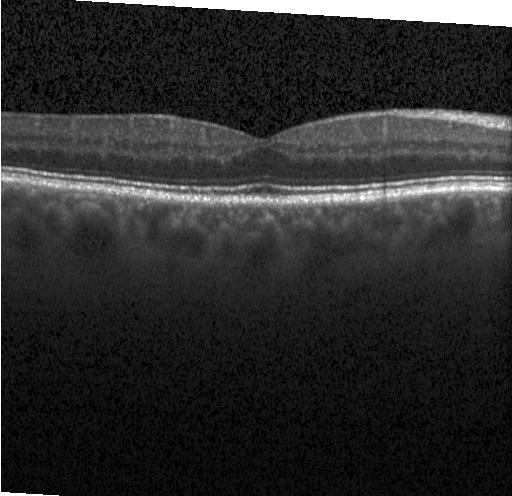 Dx: no evidence of choroidal neovascularization, diabetic macular edema, or drusen.